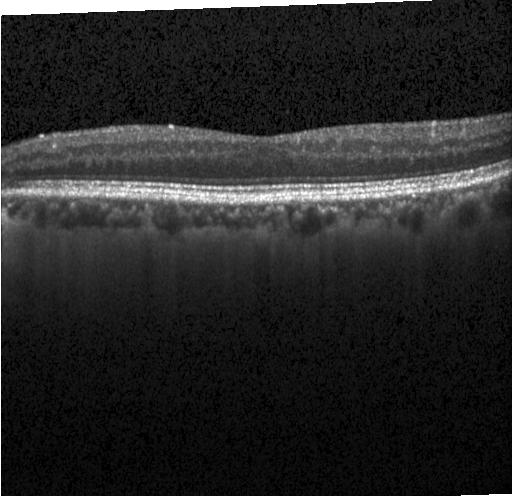

Diagnosis: no CNV, DME, or drusen.